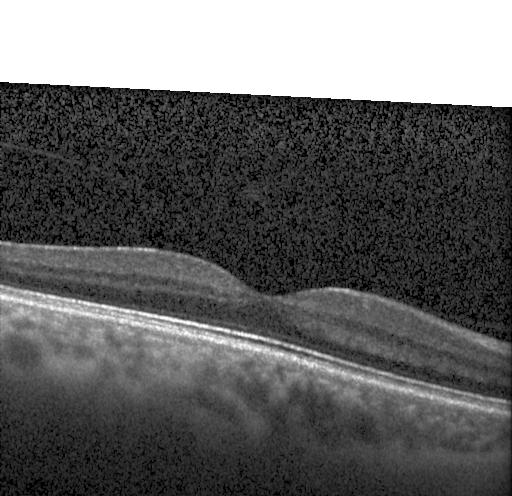

Finding: neither CNV, DME, nor drusen.